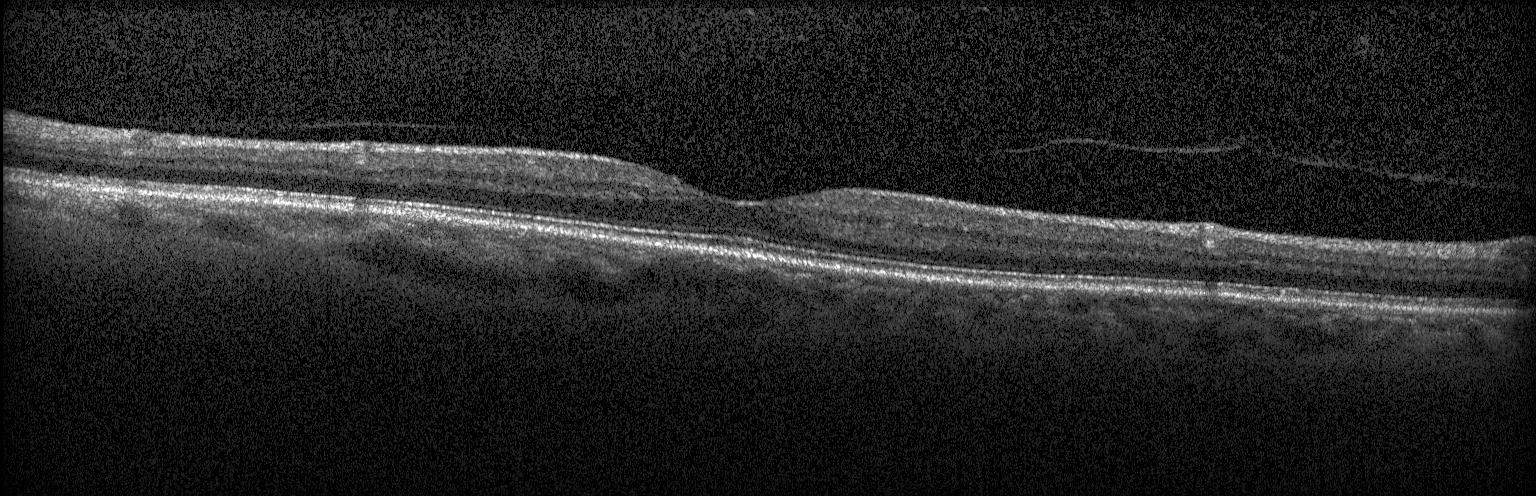 Finding: no evidence of CNV, DME, or drusen.